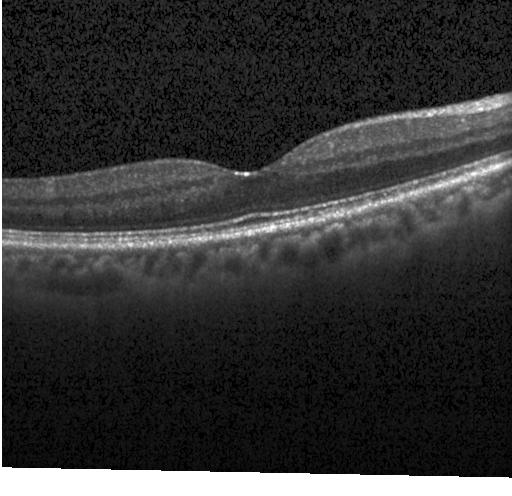 Diagnosis: no choroidal neovascularization, diabetic macular edema, or drusen.